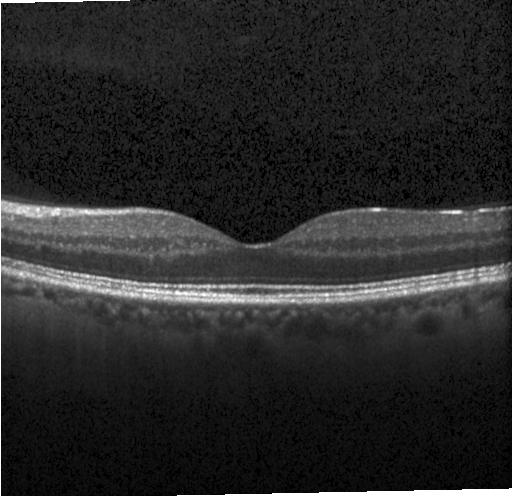 Impression: neither choroidal neovascularization, diabetic macular edema, nor drusen.